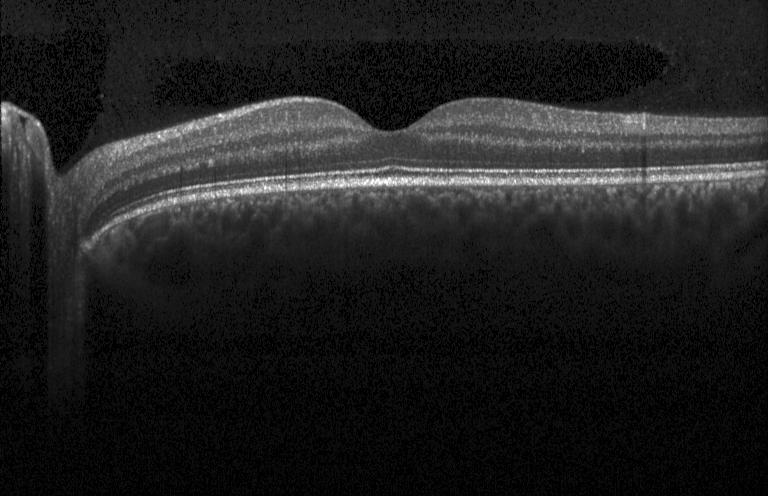

OCT scan showing no CNV, no DME, and no drusen.